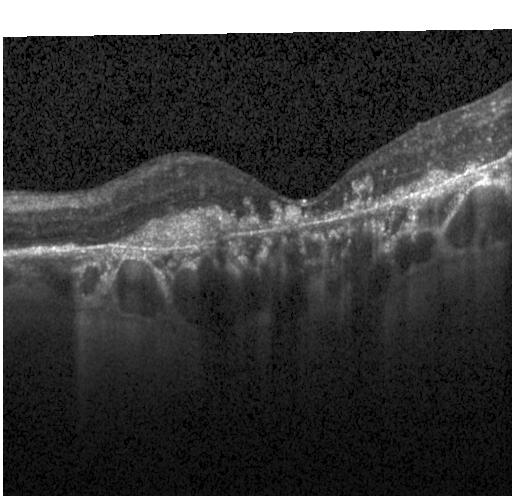

Diagnosis: choroidal neovascularization.